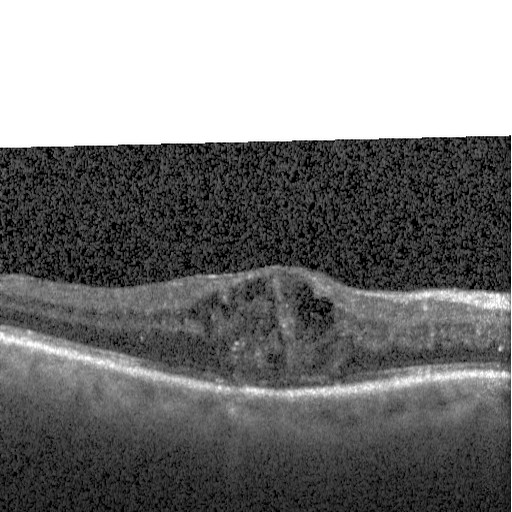

OCT B-scan
Diagnosis: diabetic macular edema.